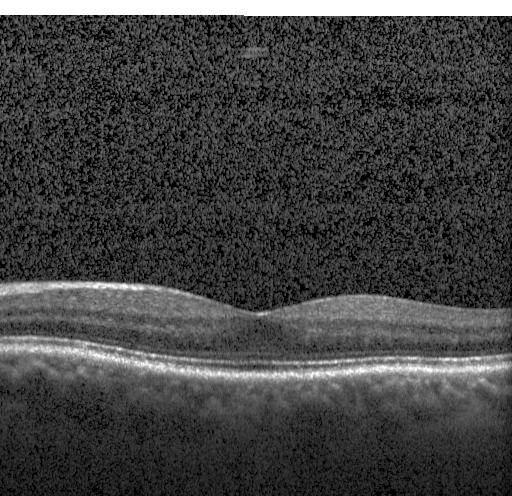
OCT B-scan — Assessment: no choroidal neovascularization, no diabetic macular edema, and no drusen.